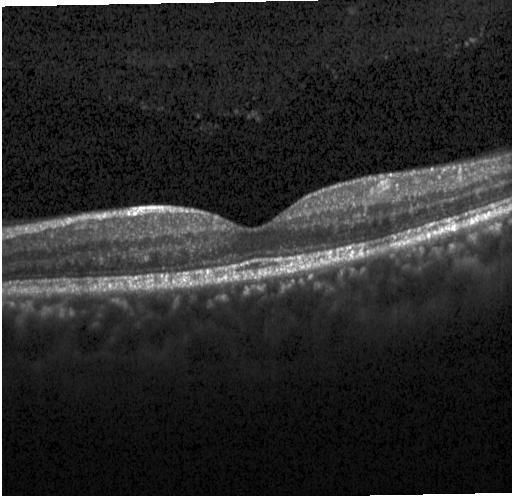 The scan shows no evidence of CNV, DME, or drusen.